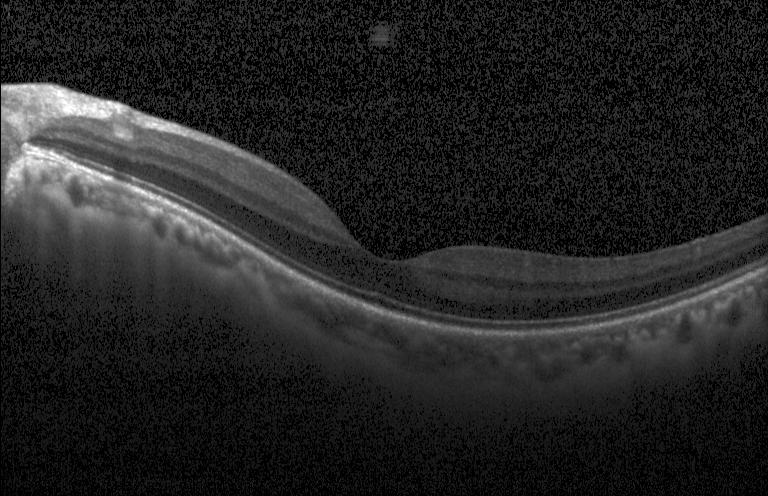

This B-scan demonstrates no choroidal neovascularization, diabetic macular edema, or drusen.